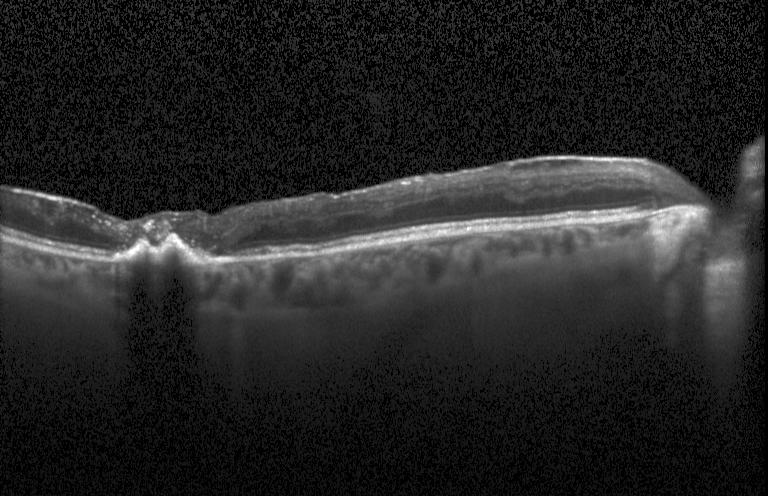
Retinal OCT cross-section
Impression: a choroidal neovascular membrane.